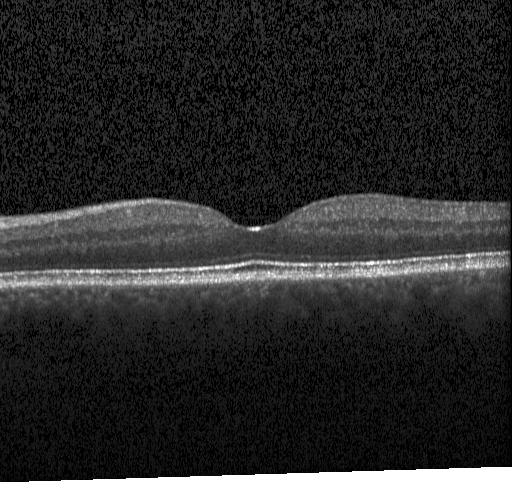
Impression: no choroidal neovascularization, no diabetic macular edema, and no drusen.